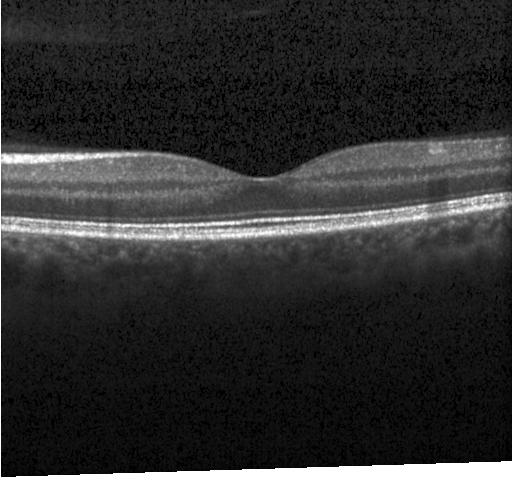
OCT line scan, spectral-domain optical coherence tomography, Heidelberg Spectralis OCT system.
Diagnosis: no evidence of choroidal neovascularization, diabetic macular edema, or drusen.